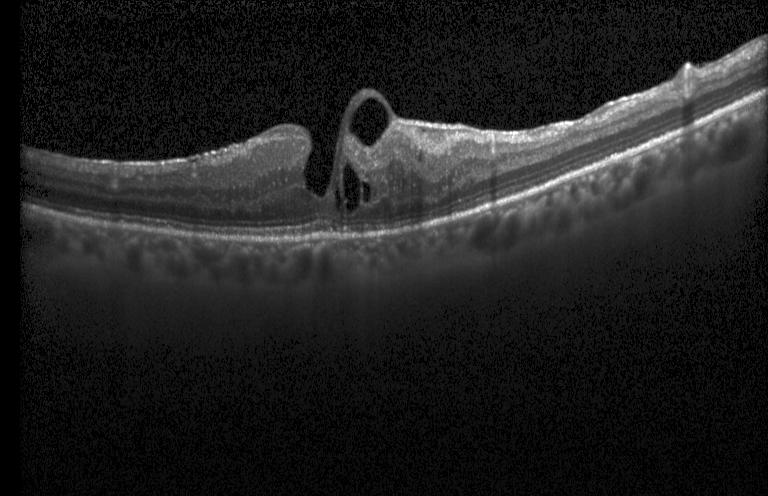
OCT B-scan. Heidelberg Spectralis. Through the macula. SD-OCT. Macular OCT: diabetic macular edema (DME).